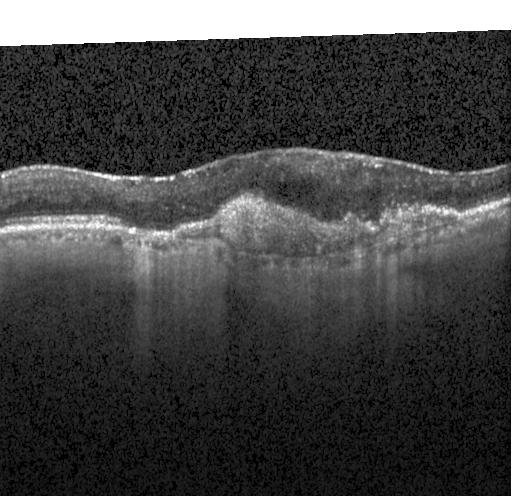
Macular OCT demonstrating choroidal neovascularization (CNV).